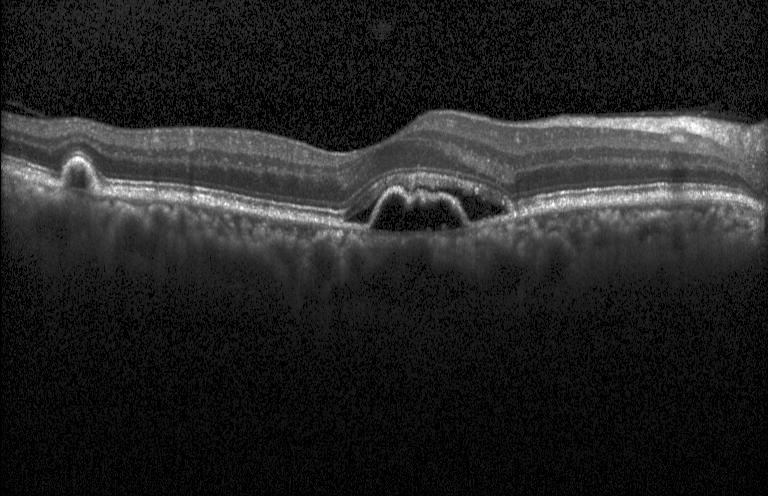 Spectral-domain optical coherence tomography. Optical coherence tomography B-scan. Through the macula. Instrument: Heidelberg Spectralis. The scan shows choroidal neovascularization.